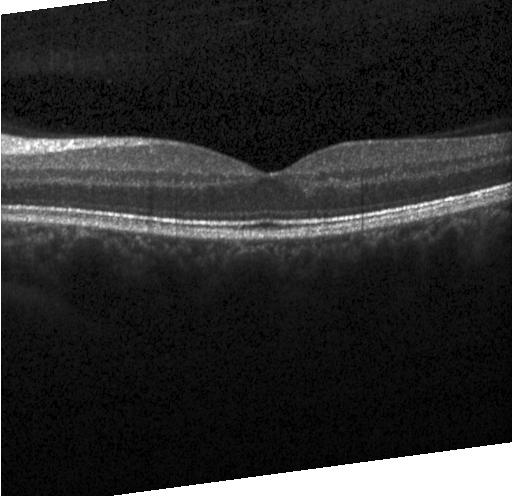 SD-OCT · OCT line scan · Heidelberg Spectralis · macular scan. Macular OCT: neither choroidal neovascularization, diabetic macular edema, nor drusen.